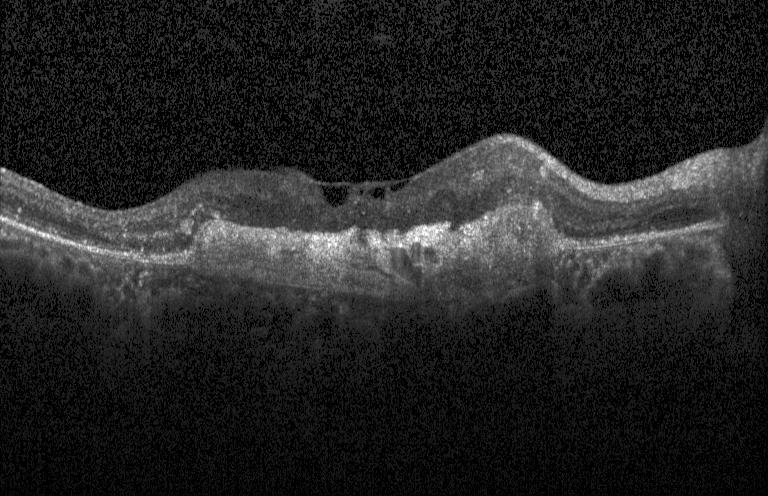

OCT line scan.
Macular OCT: CNV.